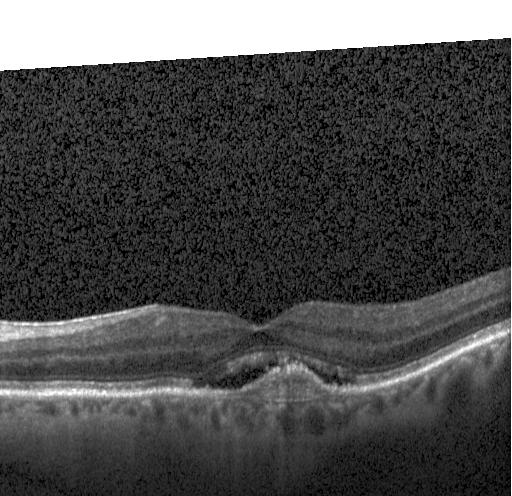
Impression: a choroidal neovascular membrane.